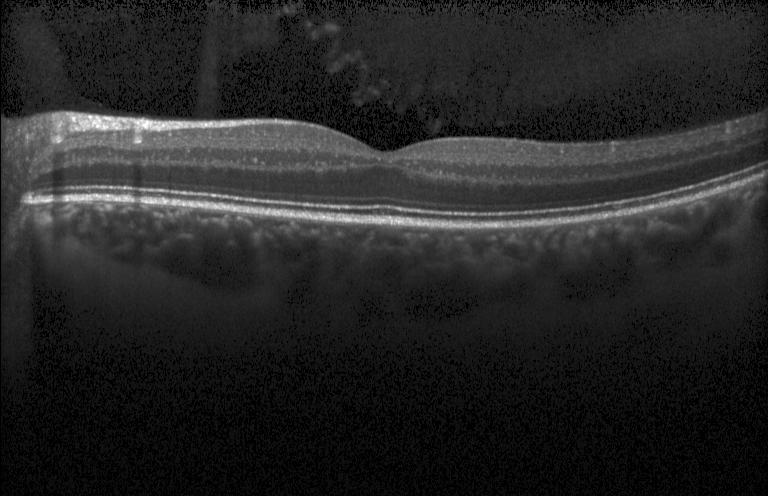 Macular OCT demonstrating no evidence of choroidal neovascularization, diabetic macular edema, or drusen.